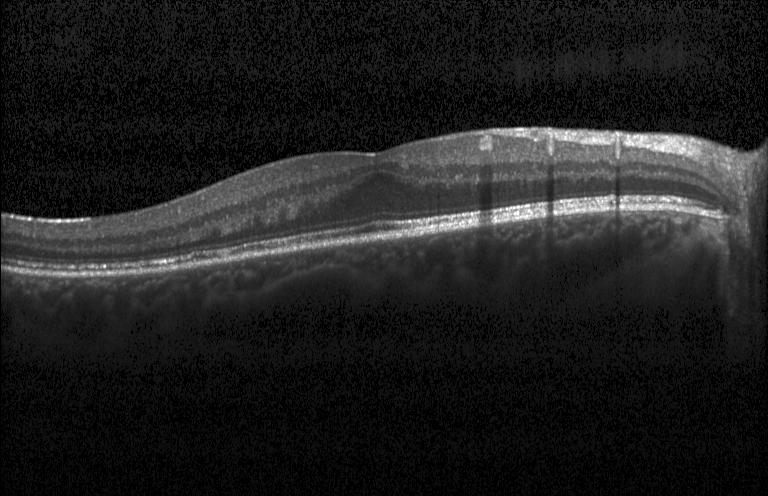 Instrument: Heidelberg Spectralis, retinal OCT B-scan, macular scan, spectral-domain optical coherence tomography
Assessment: no evidence of choroidal neovascularization, diabetic macular edema, or drusen.